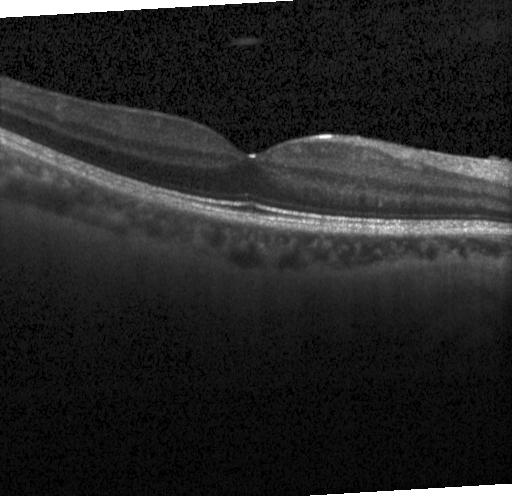

Finding: neither choroidal neovascularization, diabetic macular edema, nor drusen.